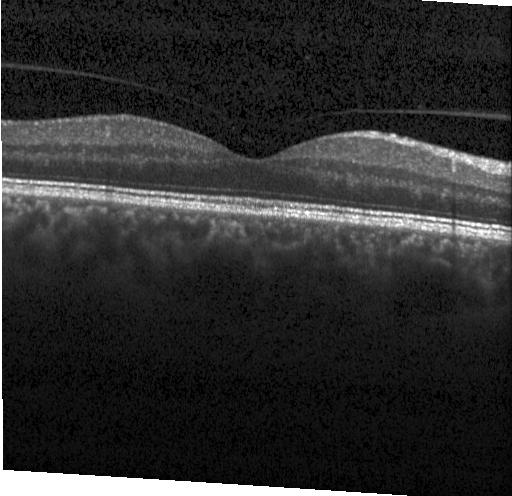

OCT scan showing no evidence of choroidal neovascularization, diabetic macular edema, or drusen.